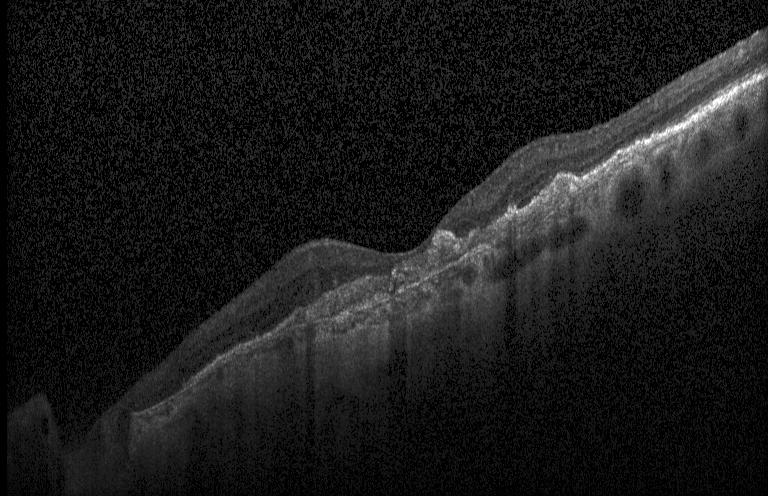

Heidelberg Spectralis OCT system. Fovea-centered. Spectral-domain OCT. OCT B-scan
Diagnosis: CNV.